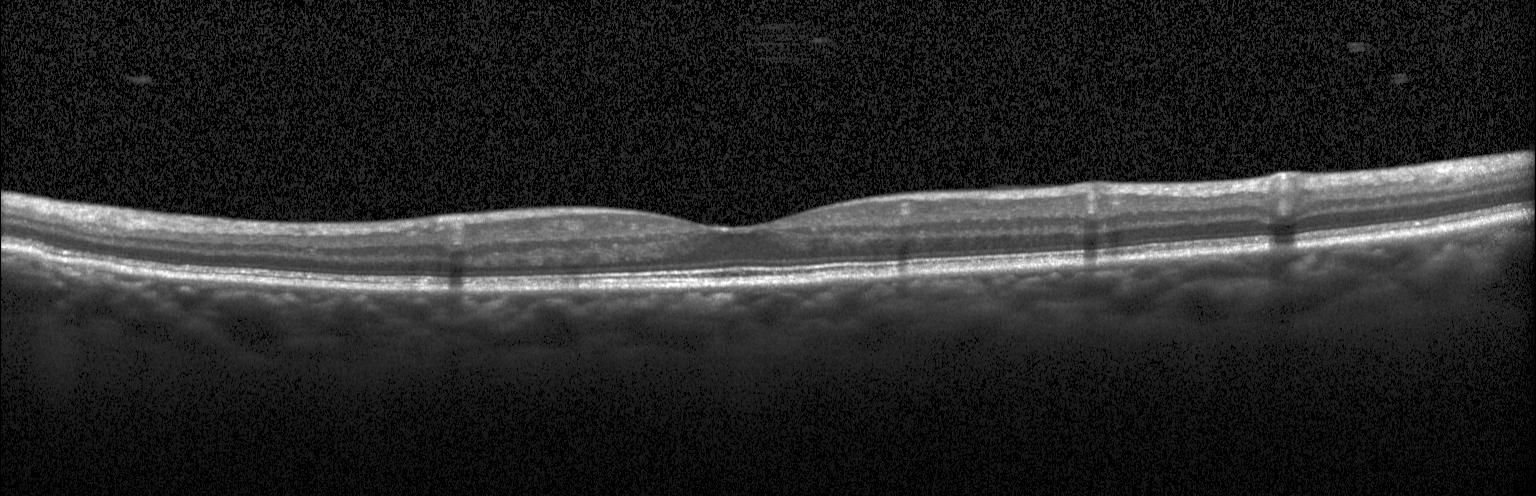

Impression: no CNV, no DME, and no drusen.